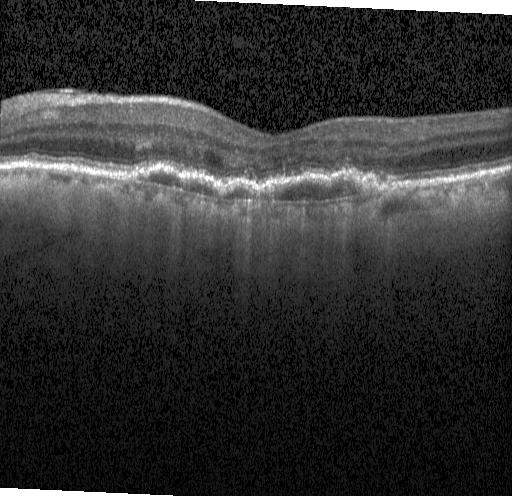 Impression: a choroidal neovascular membrane.